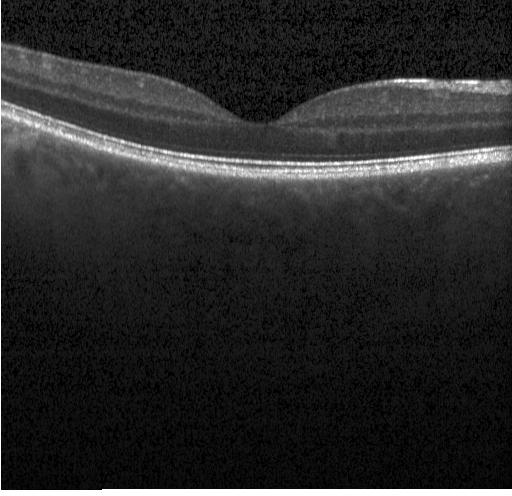
Optical coherence tomography B-scan. Finding: no evidence of choroidal neovascularization, diabetic macular edema, or drusen.